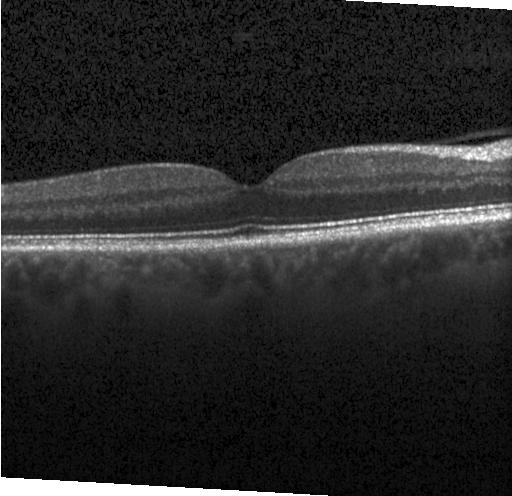

Optical coherence tomography scan — The scan shows no choroidal neovascularization, diabetic macular edema, or drusen.